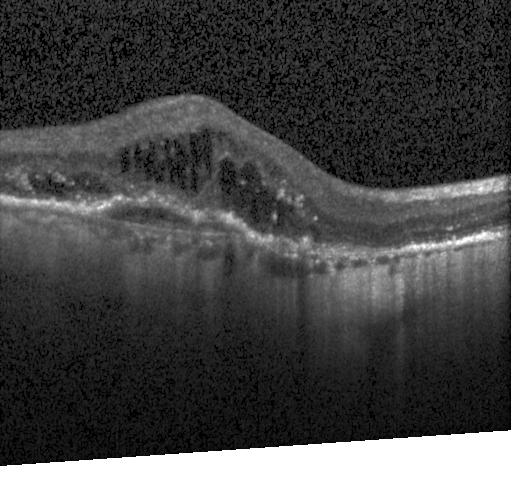 OCT B-scan
OCT finding: a choroidal neovascular membrane.